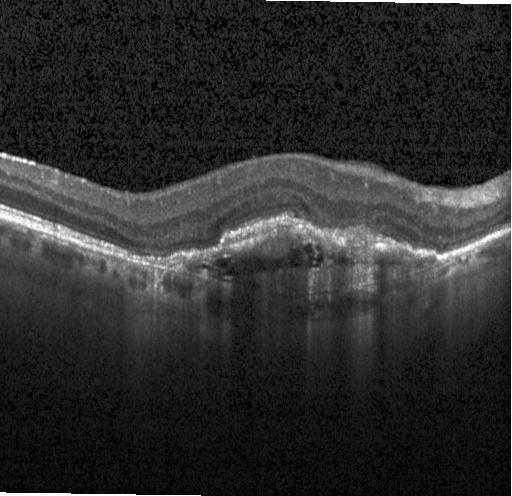

Spectral-domain OCT · horizontal scan through the fovea · instrument: Heidelberg Spectralis · OCT line scan. Assessment: choroidal neovascularization.